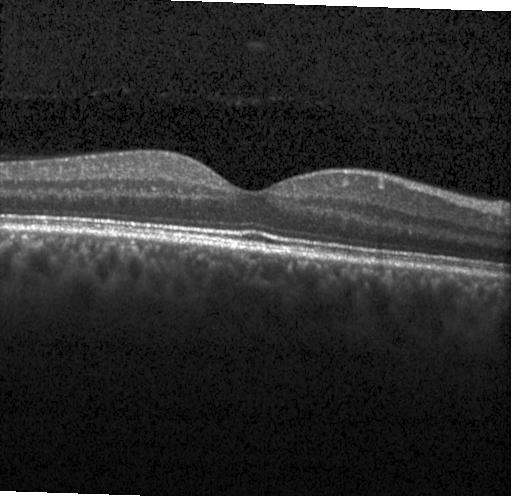

Finding: no CNV, no DME, and no drusen.